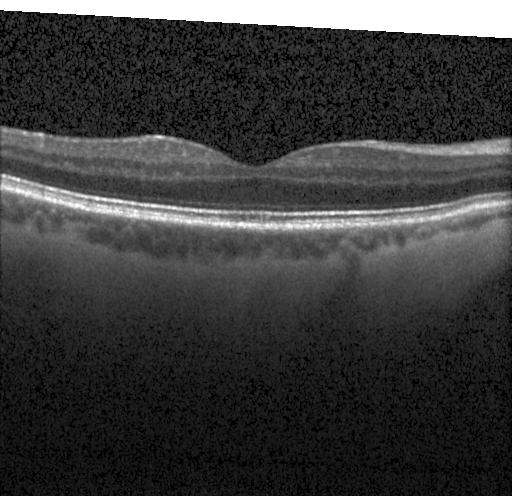
Retinal OCT B-scan.
Impression: neither choroidal neovascularization, diabetic macular edema, nor drusen.